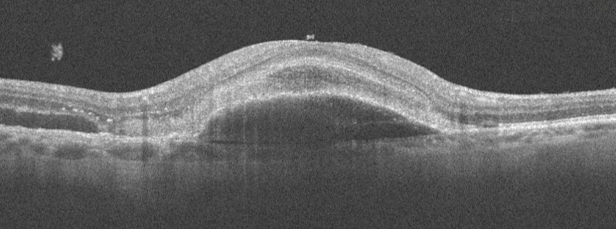 Retinal OCT cross-section showing age-related macular degeneration (AMD).